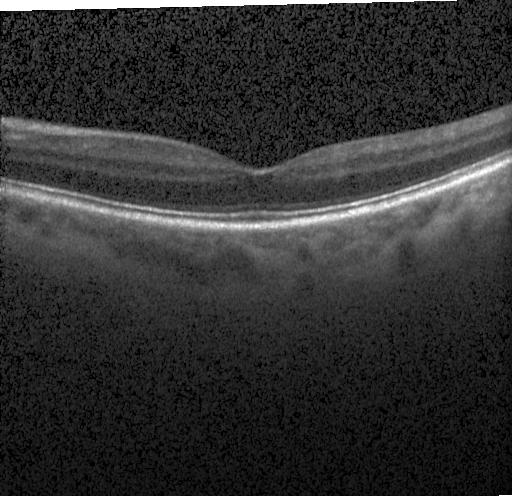
SD-OCT. Retinal OCT B-scan.
Diagnosis: neither CNV, DME, nor drusen.